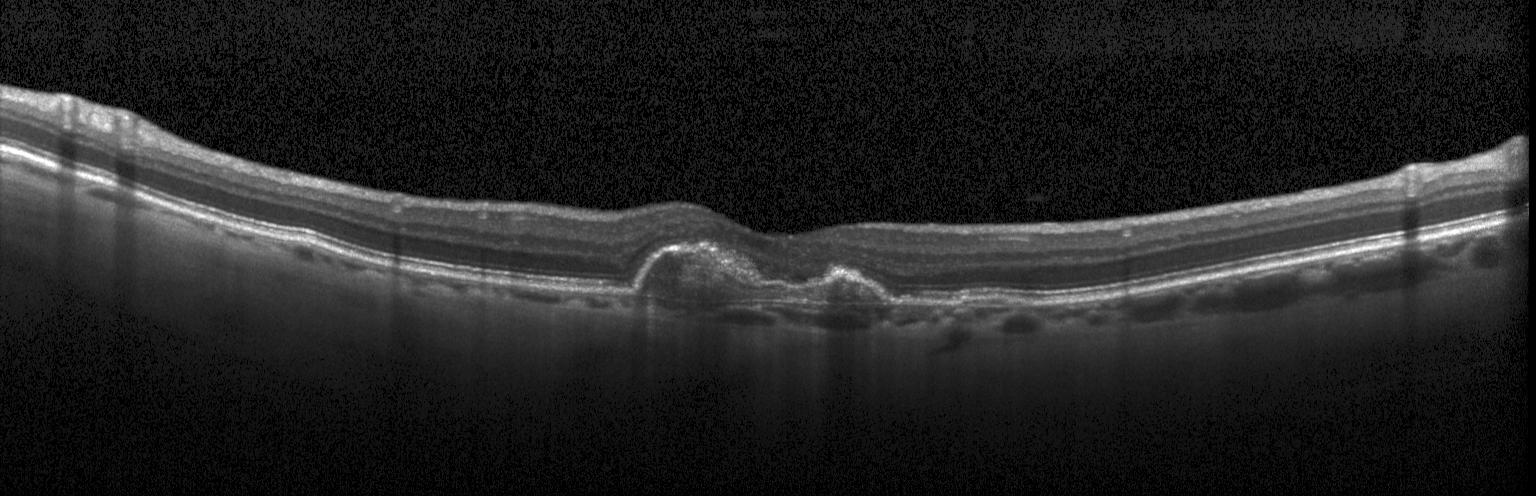
Retinal OCT cross-section · spectral-domain OCT — Assessment: CNV.